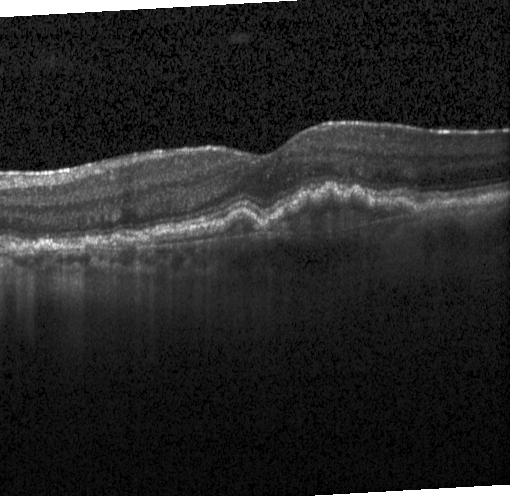

Spectral-domain OCT · Heidelberg Spectralis OCT system · OCT B-scan
Choroidal neovascularization.